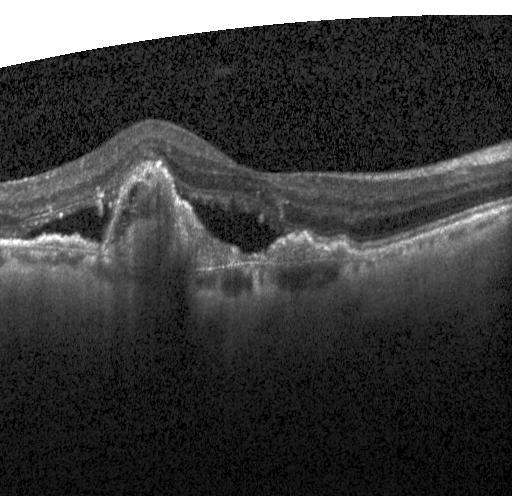
SD-OCT. Through the macula. Optical coherence tomography scan. Acquired on a Heidelberg Spectralis. Diagnosis: choroidal neovascularization (CNV).